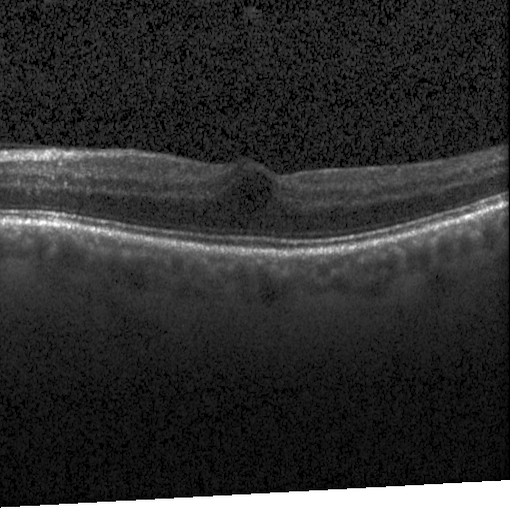
Heidelberg Spectralis OCT system · retinal OCT cross-section — Impression: diabetic macular edema (DME).